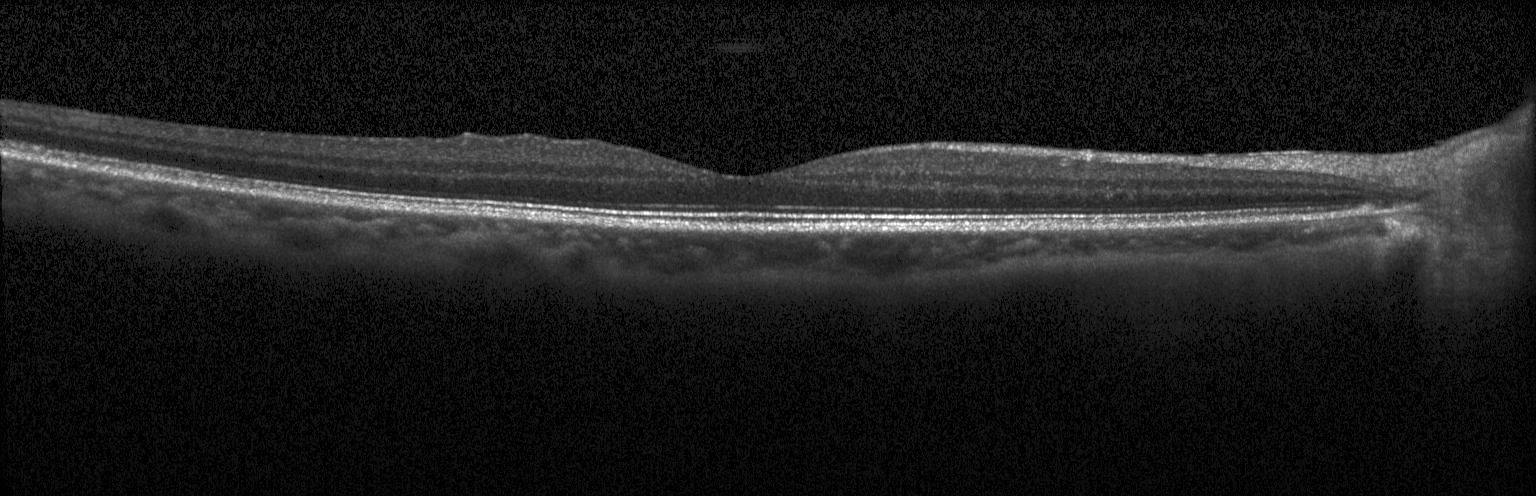

OCT B-scan, spectral-domain OCT, macular scan, acquired on a Heidelberg Spectralis. Dx: no CNV, DME, or drusen.